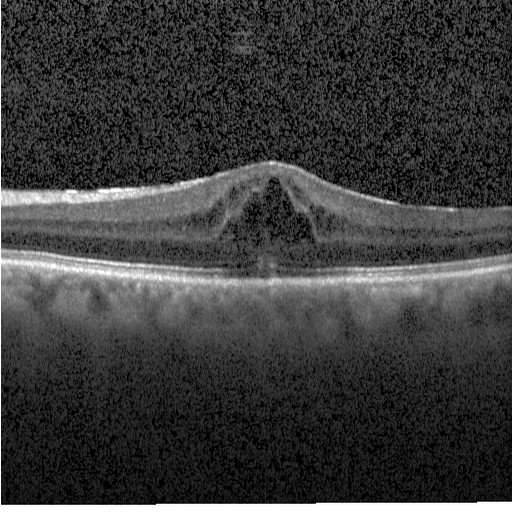

Centered on the fovea. Heidelberg Spectralis. Optical coherence tomography B-scan. Spectral-domain optical coherence tomography. Assessment: diabetic macular edema.